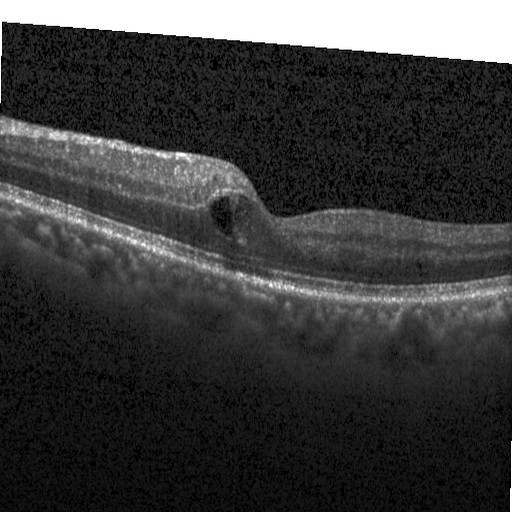
OCT finding: diabetic macular edema.